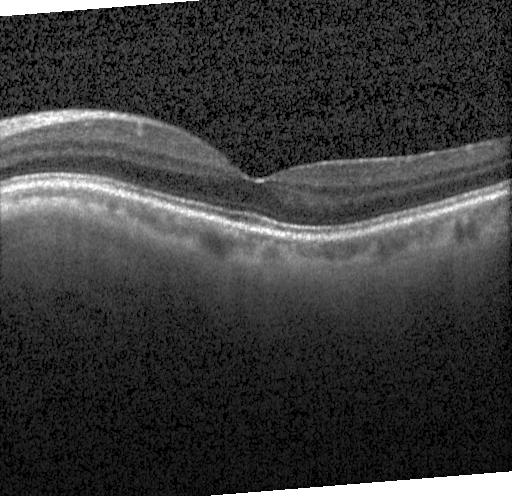

OCT B-scan.
This B-scan demonstrates no evidence of choroidal neovascularization, diabetic macular edema, or drusen.